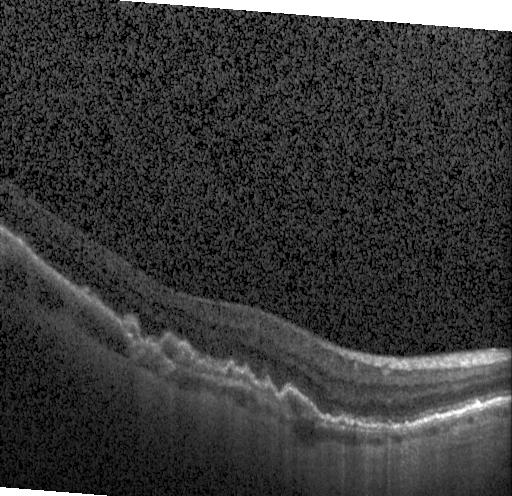
Impression: a choroidal neovascular membrane.